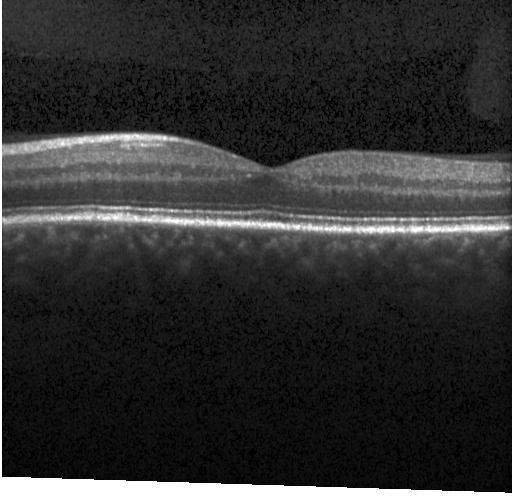 OCT finding: no choroidal neovascularization, no diabetic macular edema, and no drusen.